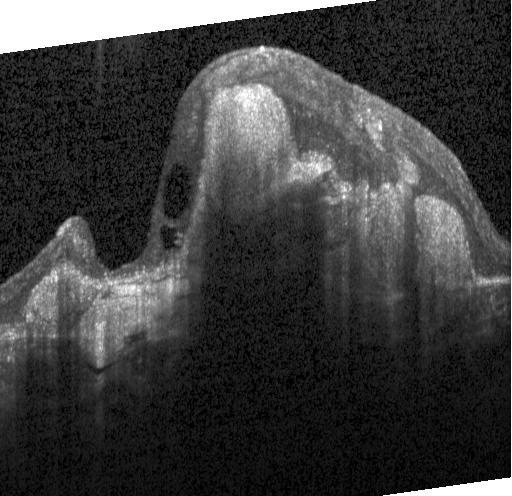
Horizontal scan through the fovea; OCT B-scan — Diagnosis: choroidal neovascularization.